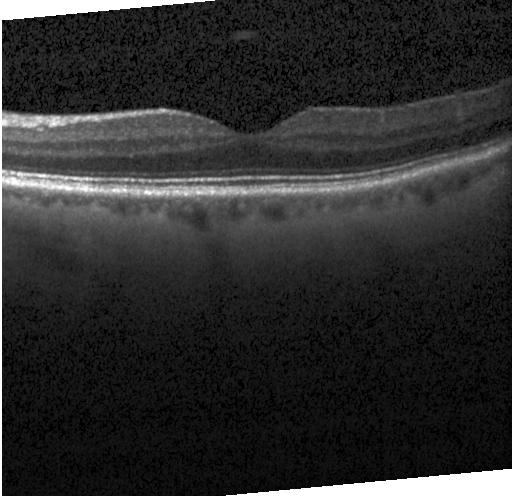

Diagnosis: neither choroidal neovascularization, diabetic macular edema, nor drusen.